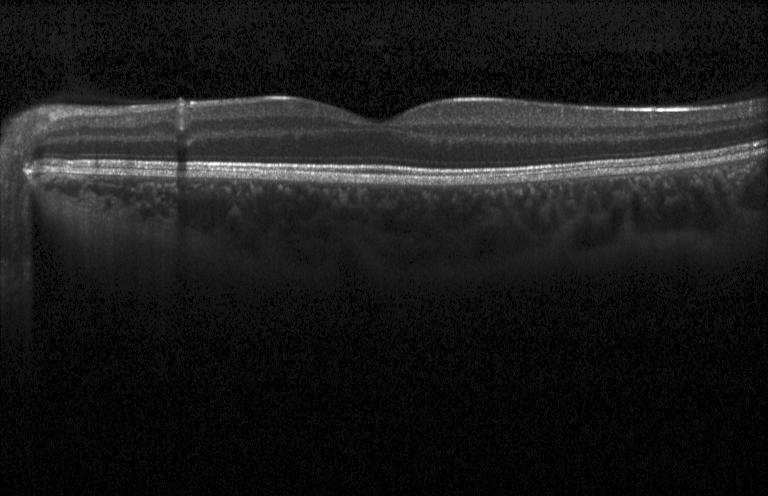

OCT finding: no choroidal neovascularization, no diabetic macular edema, and no drusen.